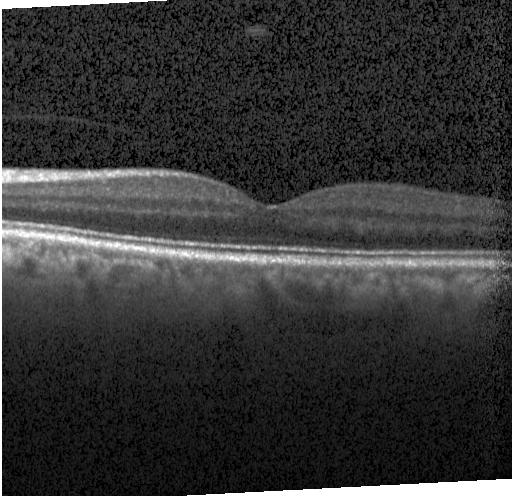

OCT line scan. Spectral-domain OCT
No evidence of CNV, DME, or drusen.